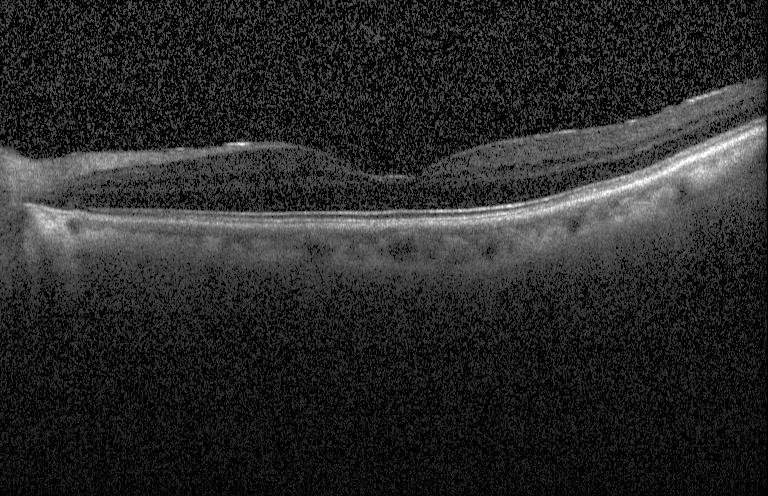
OCT scan showing no choroidal neovascularization, no diabetic macular edema, and no drusen.